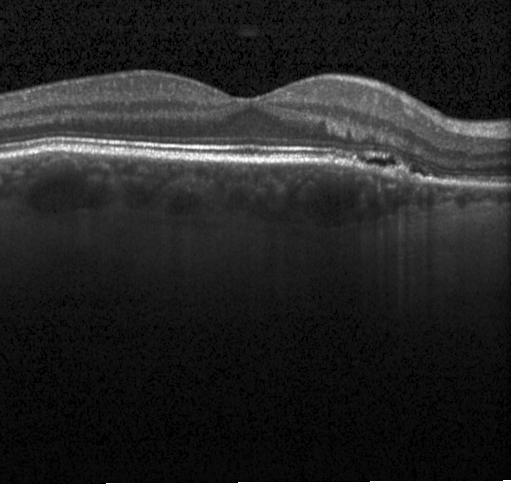

Macular OCT demonstrating CNV.